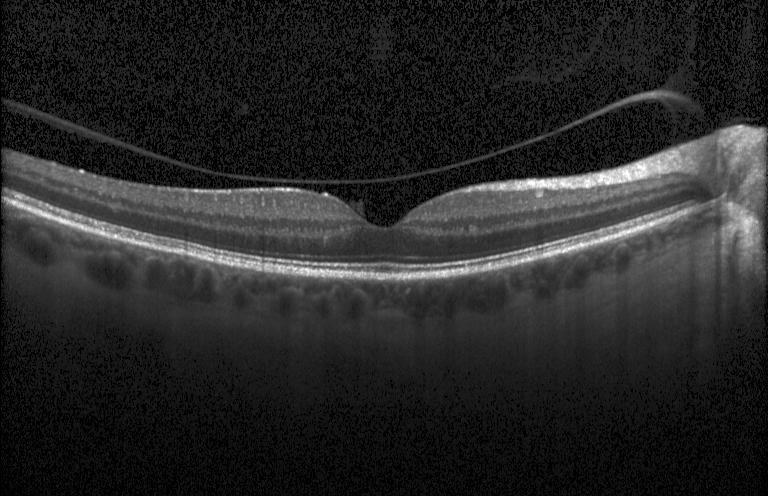

The scan shows no evidence of choroidal neovascularization, diabetic macular edema, or drusen.